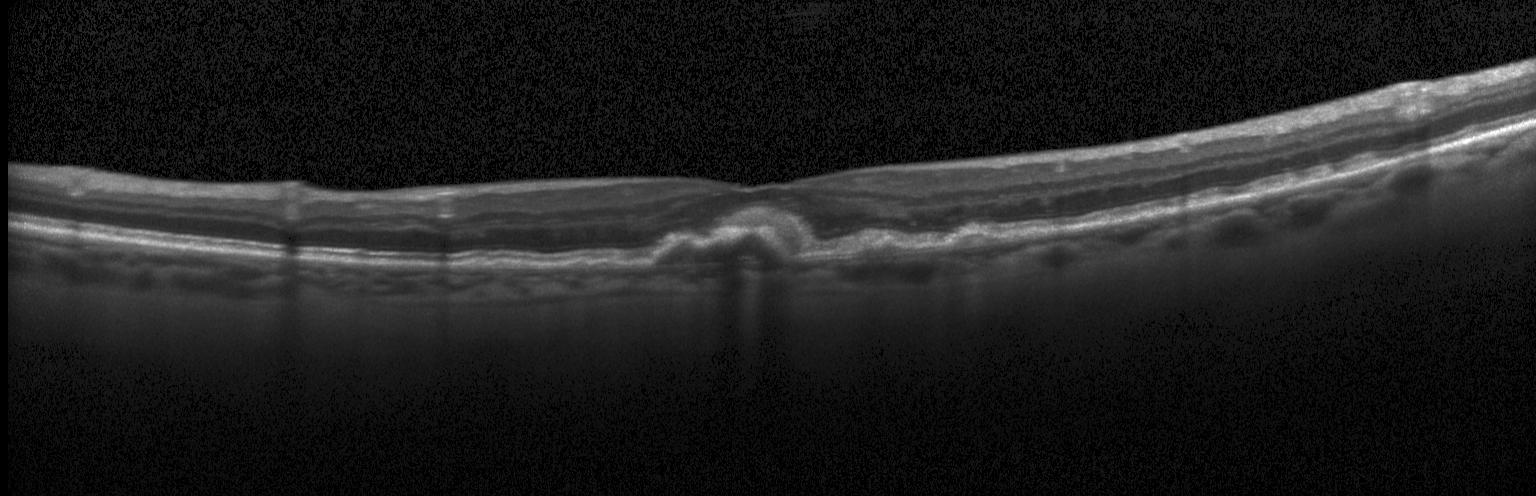
OCT line scan. SD-OCT. Fovea-centered — Impression: a choroidal neovascular membrane.